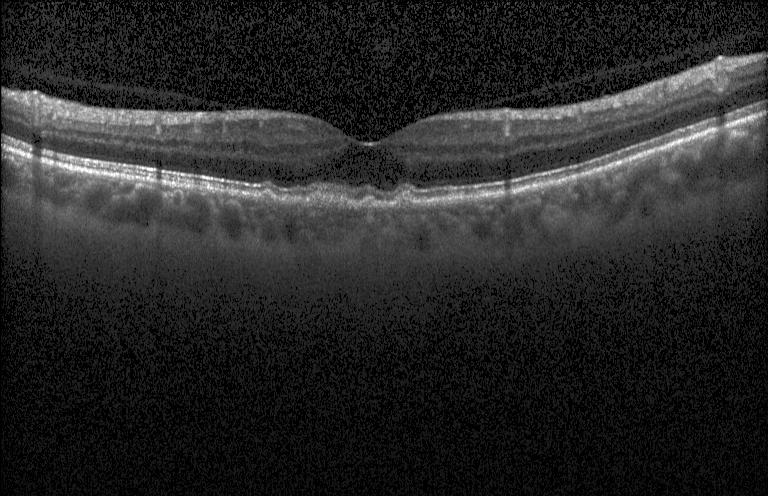

Macular OCT: sub-RPE drusenoid deposits.